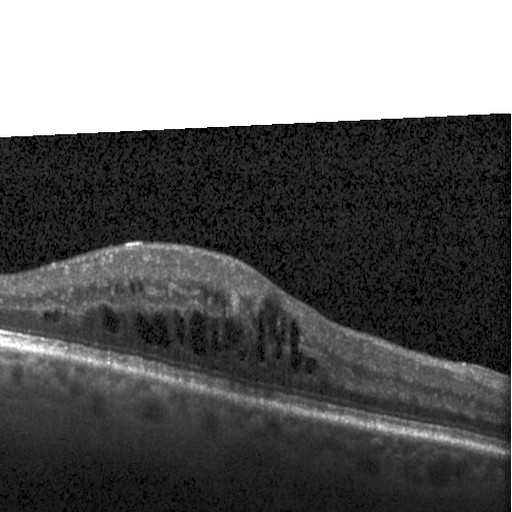 Instrument: Heidelberg Spectralis · fovea-centered · optical coherence tomography scan · spectral-domain OCT. Assessment: DME.